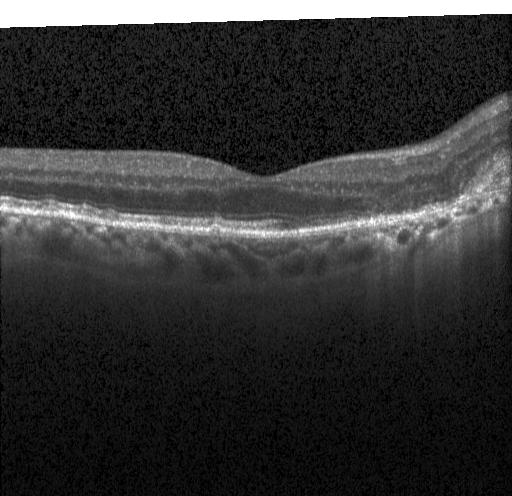
OCT B-scan — OCT finding: a choroidal neovascular membrane.